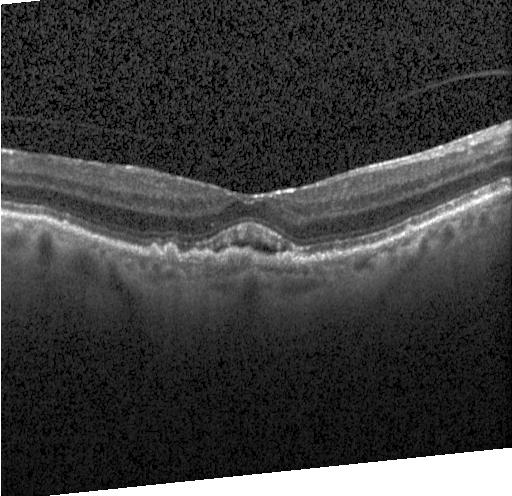

Through the macula · retinal OCT B-scan · spectral-domain optical coherence tomography · instrument: Heidelberg Spectralis. Macular OCT: a choroidal neovascular membrane.